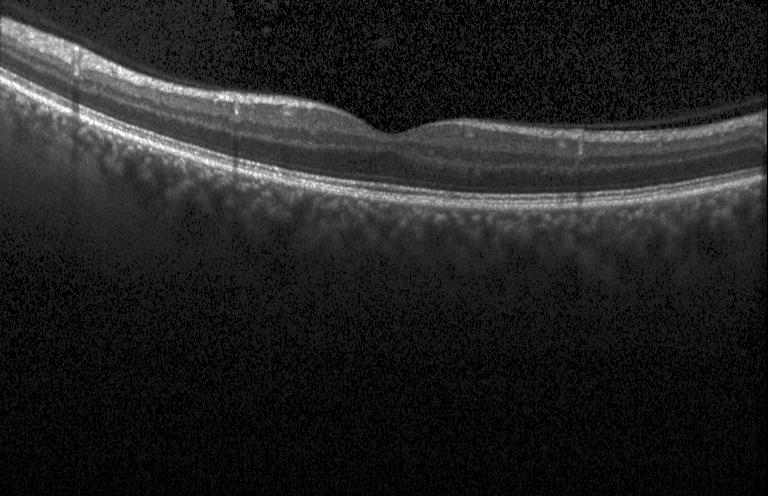 Diagnosis: neither choroidal neovascularization, diabetic macular edema, nor drusen.